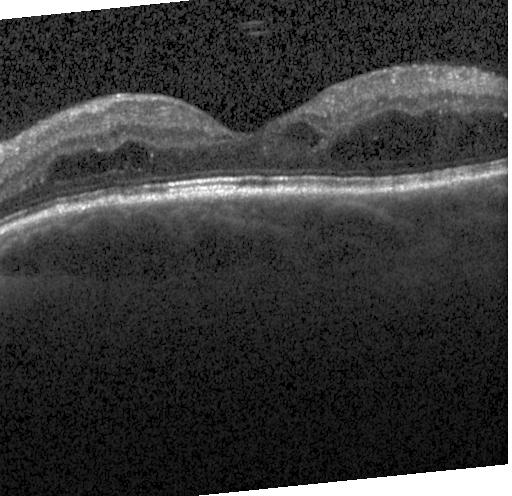

OCT finding: diabetic macular edema (DME).